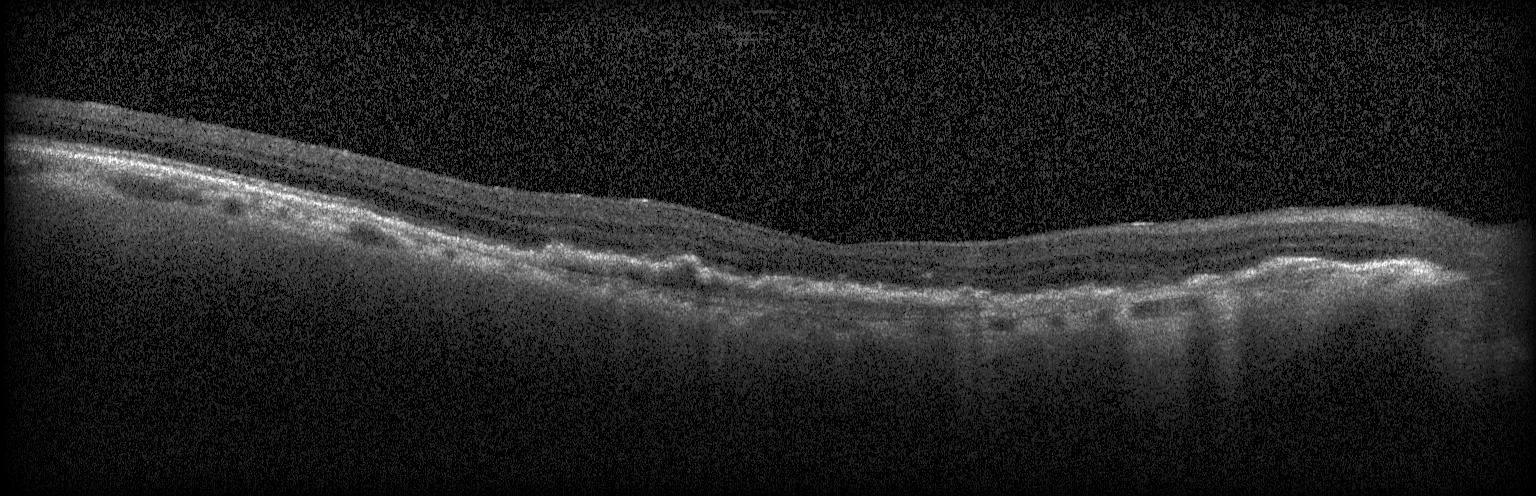
Centered on the fovea, retinal OCT B-scan
Choroidal neovascularization (CNV).